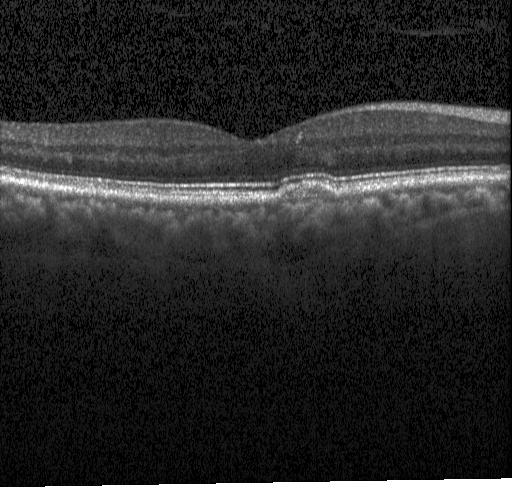 Retinal OCT B-scan · through the macula
Dx: sub-RPE drusenoid deposits.